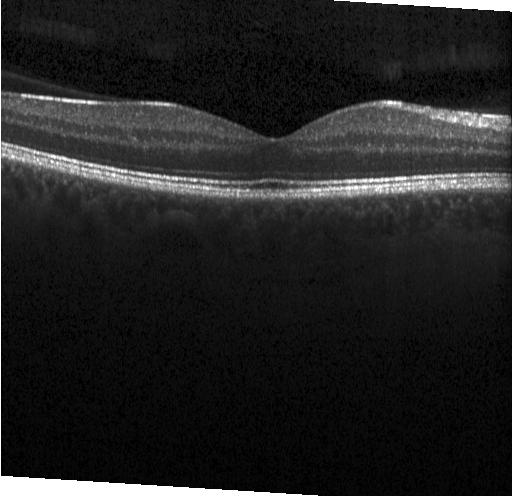 Spectral-domain OCT B-scan: no evidence of choroidal neovascularization, diabetic macular edema, or drusen.